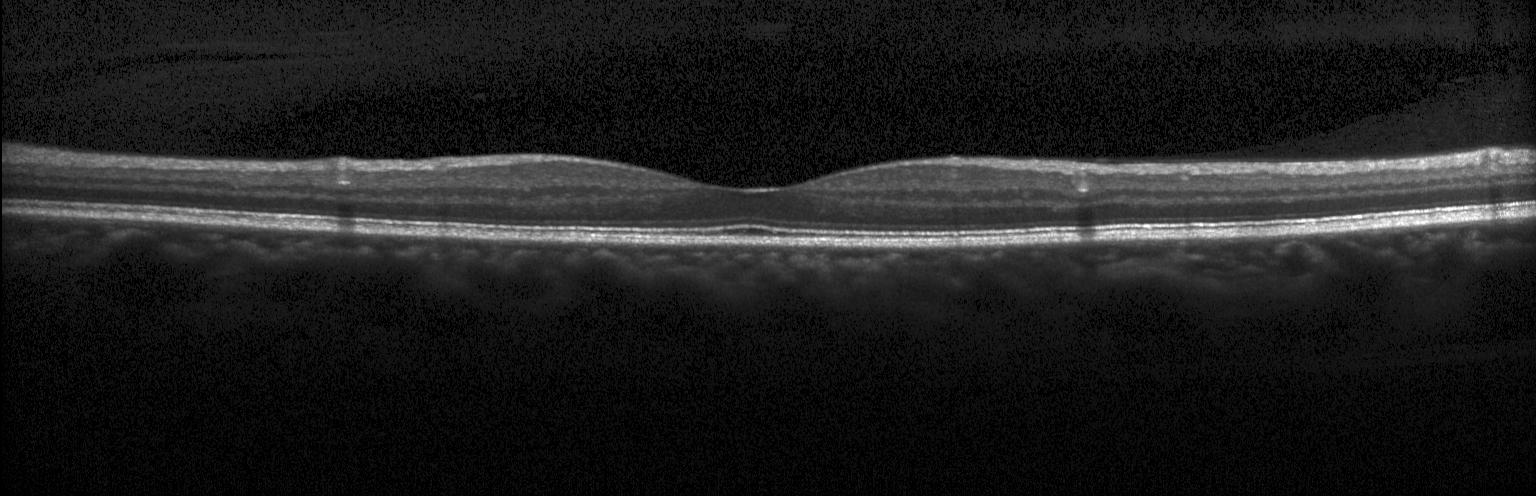
Spectral-domain OCT · OCT B-scan · Heidelberg Spectralis OCT system · macular scan
The scan shows no choroidal neovascularization, diabetic macular edema, or drusen.